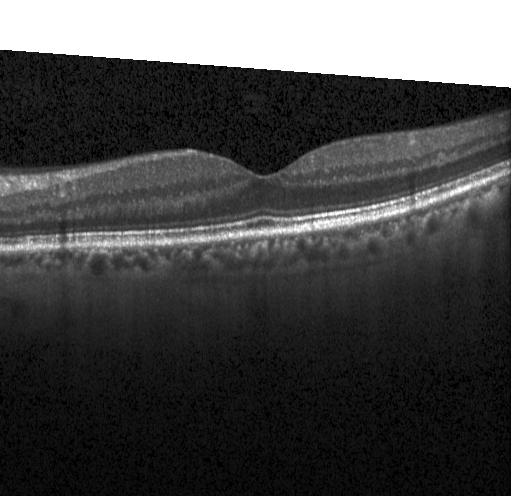

Retinal OCT B-scan. Spectral-domain optical coherence tomography
No evidence of CNV, DME, or drusen.